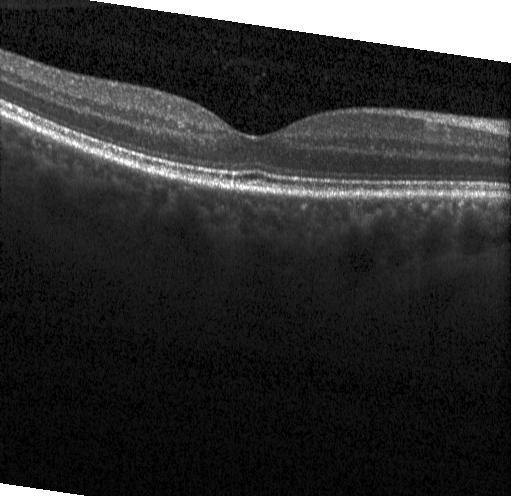 Heidelberg Spectralis · optical coherence tomography B-scan · macular scan · spectral-domain optical coherence tomography — No evidence of choroidal neovascularization, diabetic macular edema, or drusen.